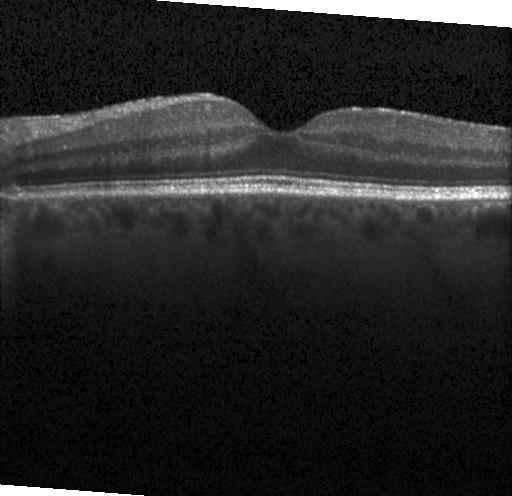
Retinal OCT B-scan · through the macula — This B-scan demonstrates neither choroidal neovascularization, diabetic macular edema, nor drusen.